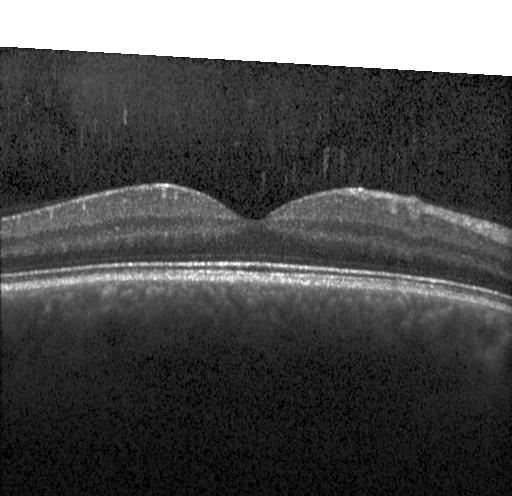

Finding: no CNV, no DME, and no drusen.